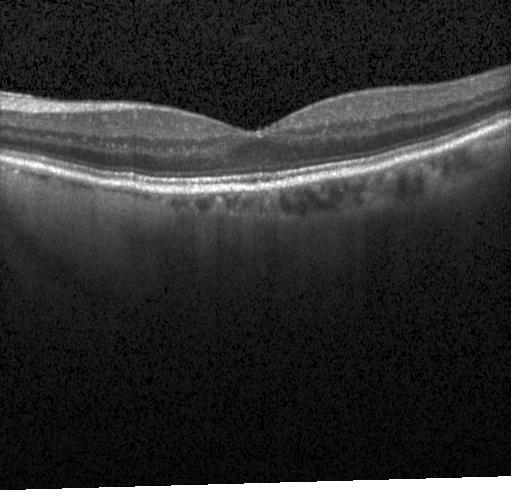 The scan shows no CNV, DME, or drusen.